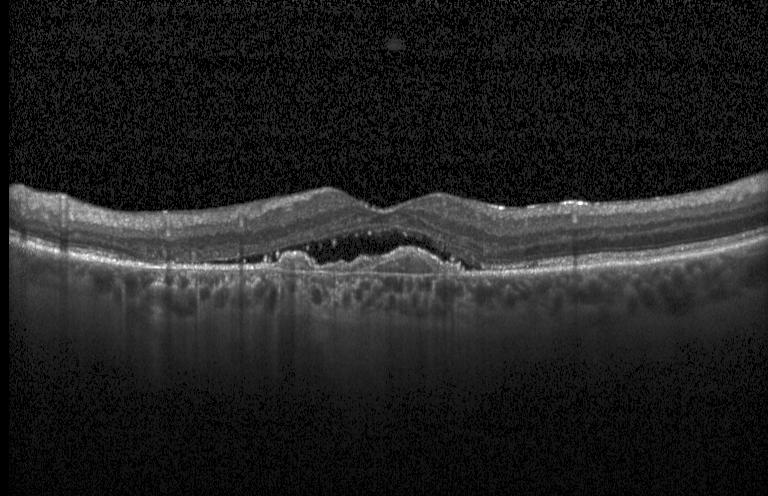 Heidelberg Spectralis OCT system. Retinal OCT cross-section. Centered on the fovea. Assessment: choroidal neovascularization.